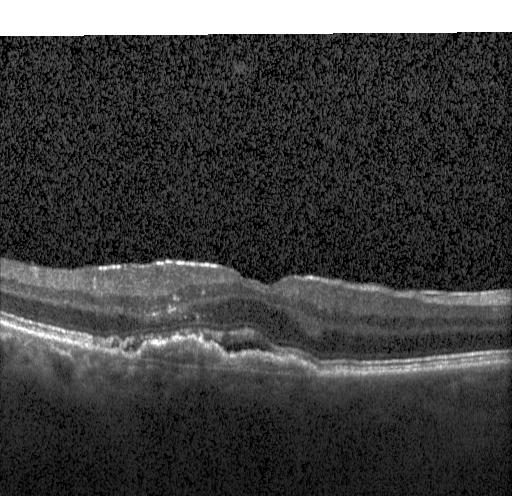

Optical coherence tomography B-scan. Impression: choroidal neovascularization.